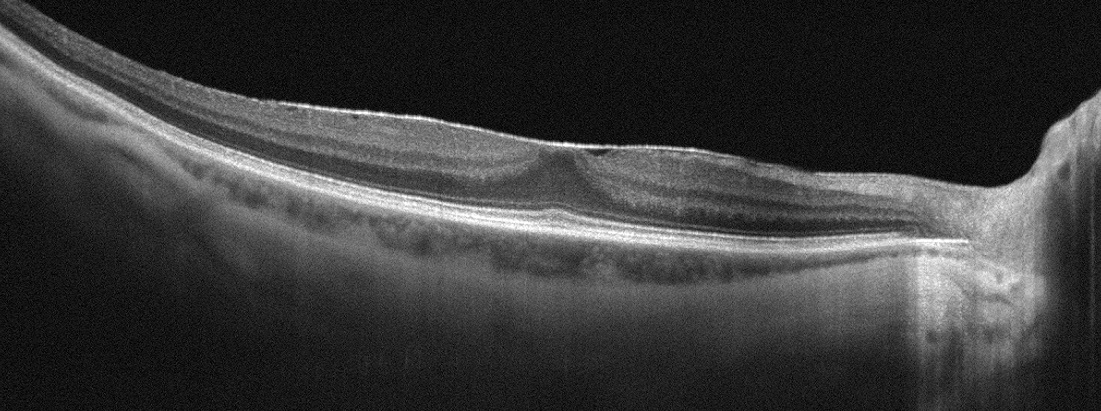 Retinal OCT cross-section · fovea-centered.
ERM.